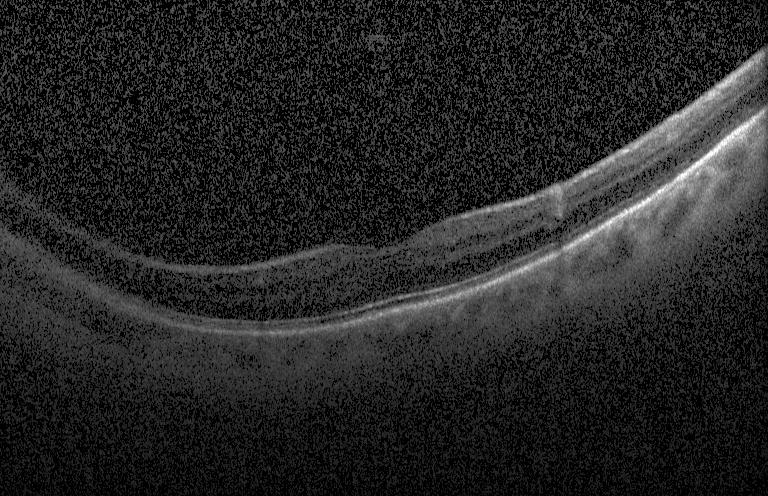 Through the macula · OCT B-scan — Dx: no CNV, DME, or drusen.